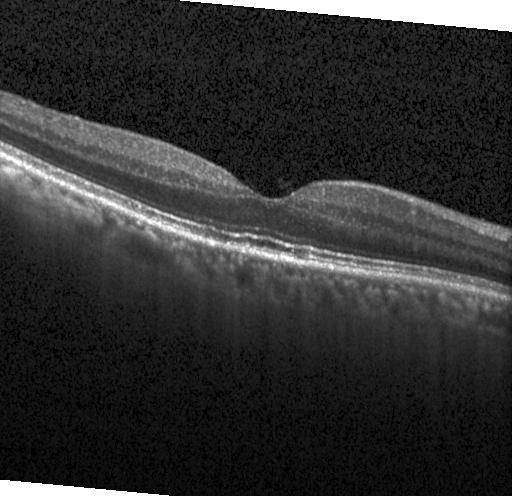

Macular OCT demonstrating no CNV, no DME, and no drusen.